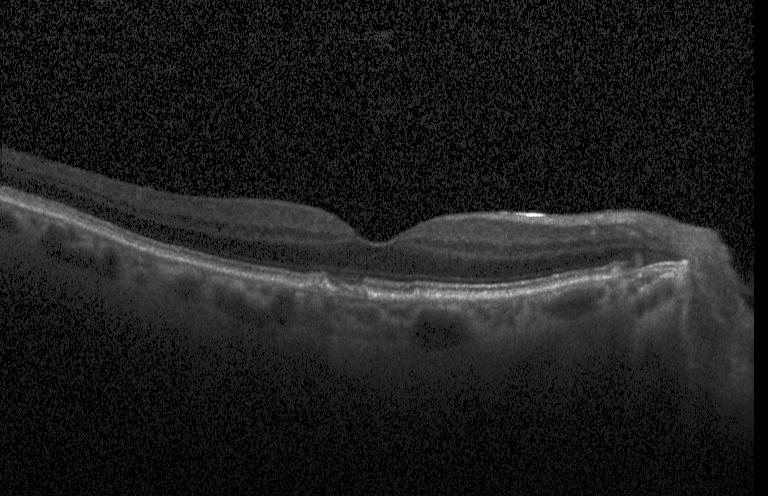 Diagnosis: drusen.